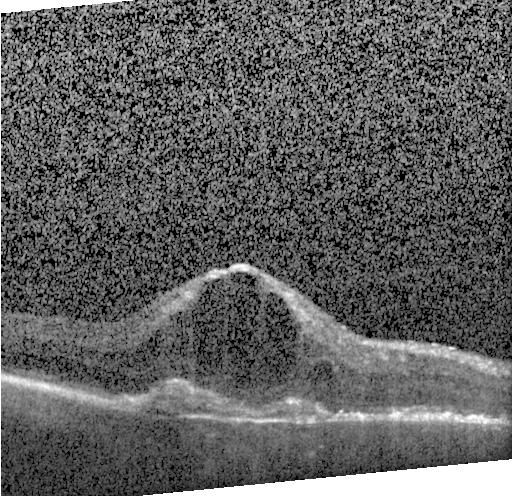
OCT B-scan · acquired on a Heidelberg Spectralis.
This B-scan demonstrates a choroidal neovascular membrane.